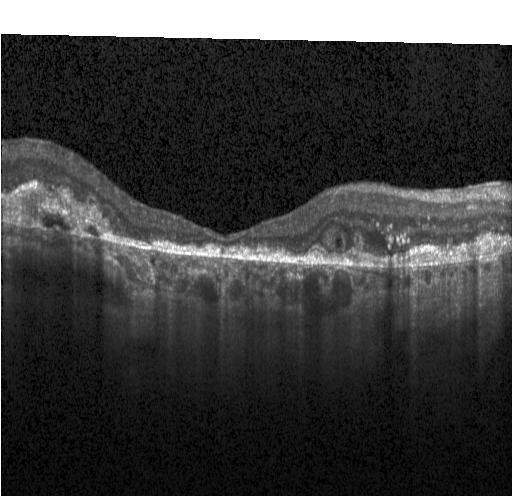 Finding: CNV.